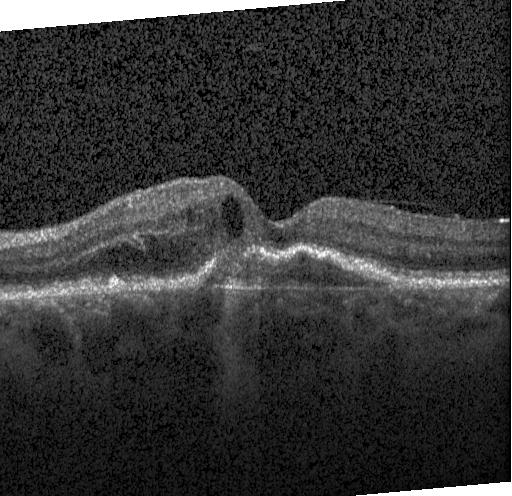
Retinal OCT B-scan, SD-OCT, centered on the fovea — Impression: CNV.